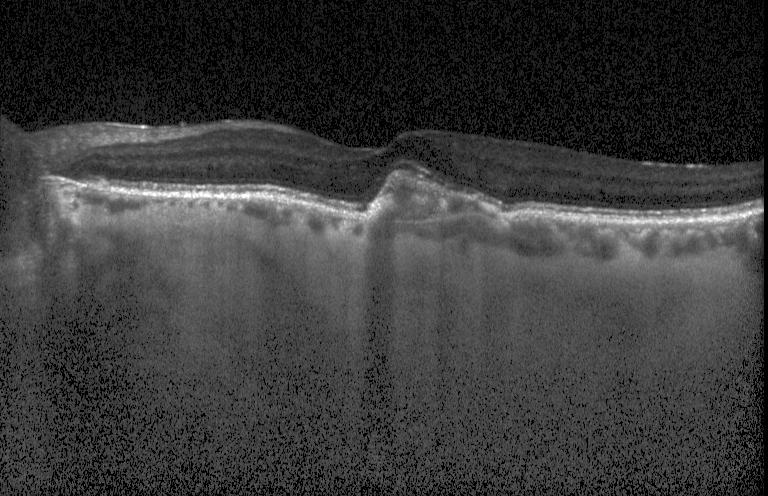

Optical coherence tomography scan. SD-OCT. OCT finding: CNV.